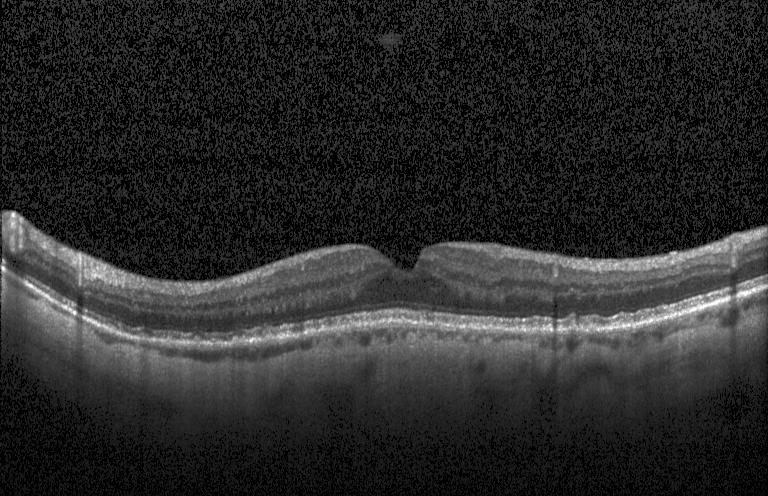
Sub-RPE drusenoid deposits.